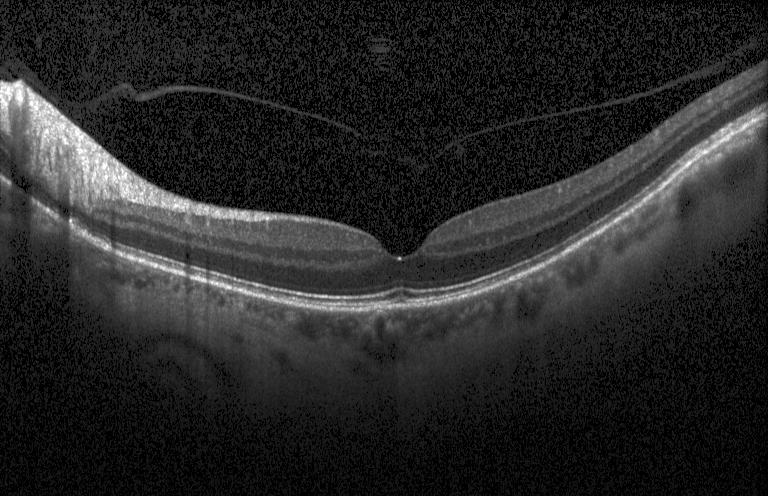

Heidelberg Spectralis. Centered on the fovea. OCT line scan. Spectral-domain optical coherence tomography.
Diagnosis: no CNV, no DME, and no drusen.